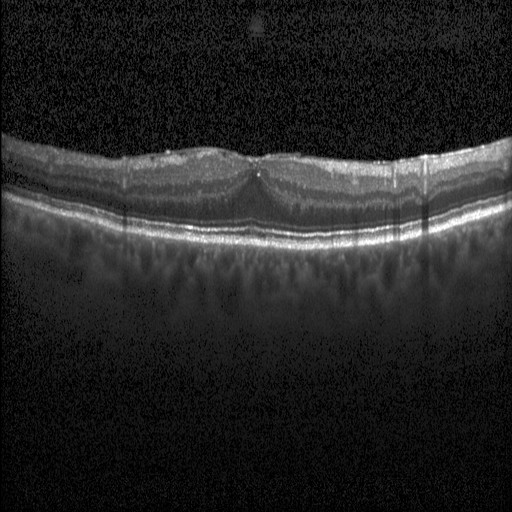
Macular OCT: diabetic macular edema.